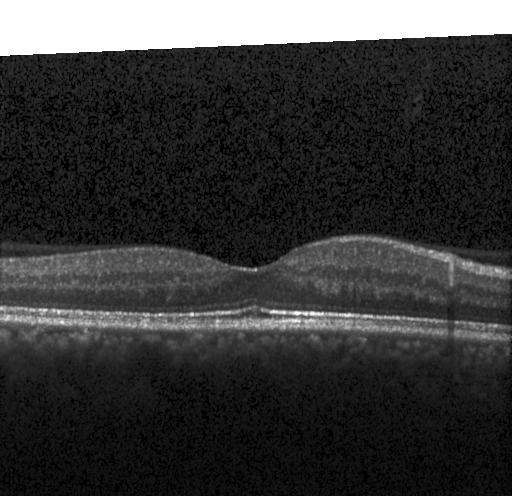
No evidence of choroidal neovascularization, diabetic macular edema, or drusen.